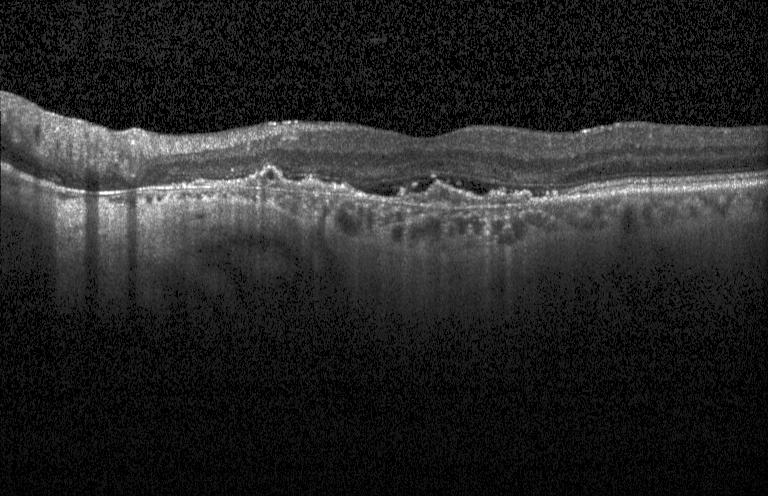 Macular OCT: choroidal neovascularization.